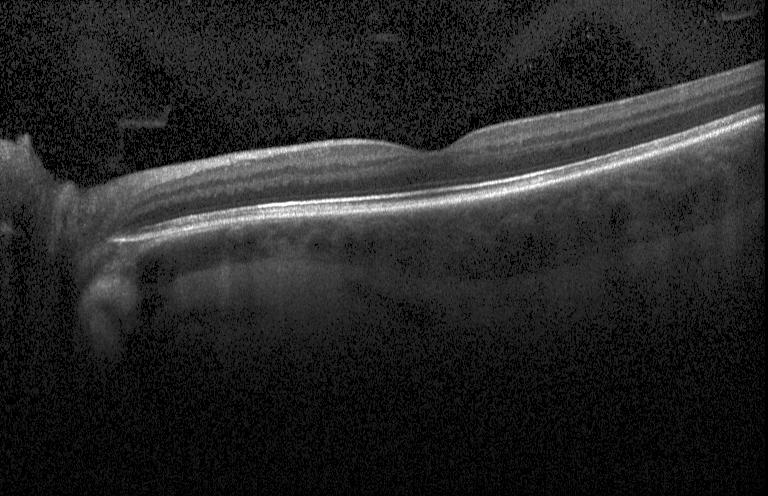

Fovea-centered · retinal OCT cross-section
Finding: no choroidal neovascularization, diabetic macular edema, or drusen.